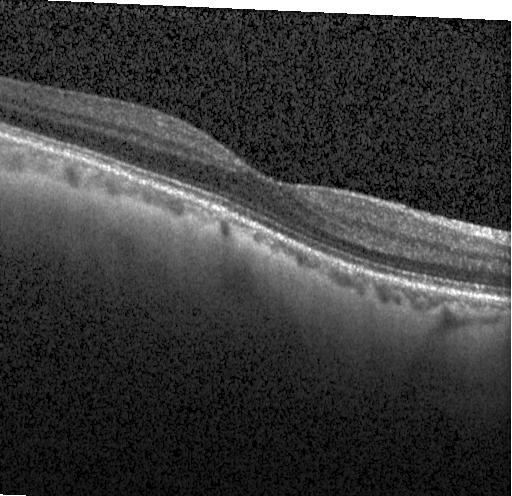
SD-OCT, Heidelberg Spectralis OCT system, fovea-centered, retinal OCT cross-section. Impression: neither CNV, DME, nor drusen.